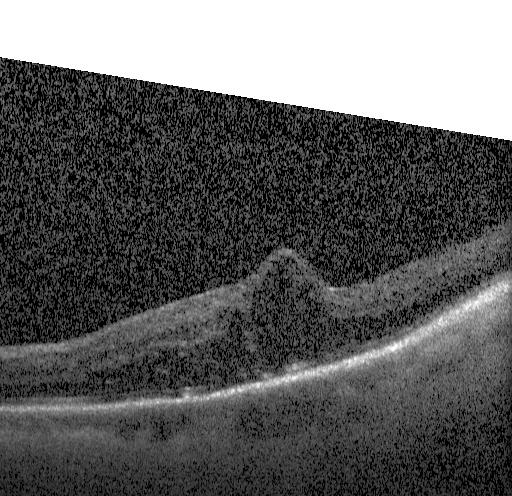
Retinal OCT cross-section. Fovea-centered. SD-OCT. Heidelberg Spectralis — OCT finding: diabetic macular edema.